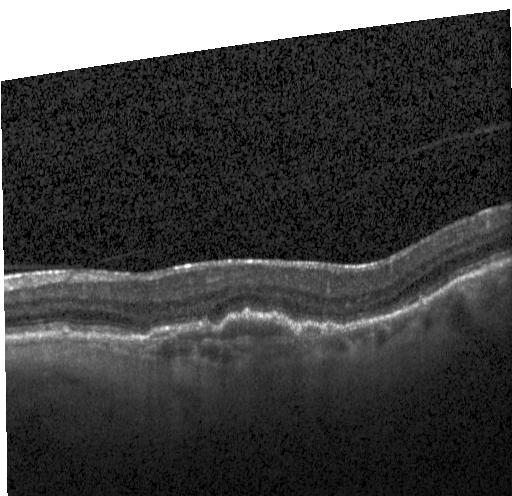
Macular scan. Retinal OCT B-scan. Acquired on a Heidelberg Spectralis — Dx: a choroidal neovascular membrane.